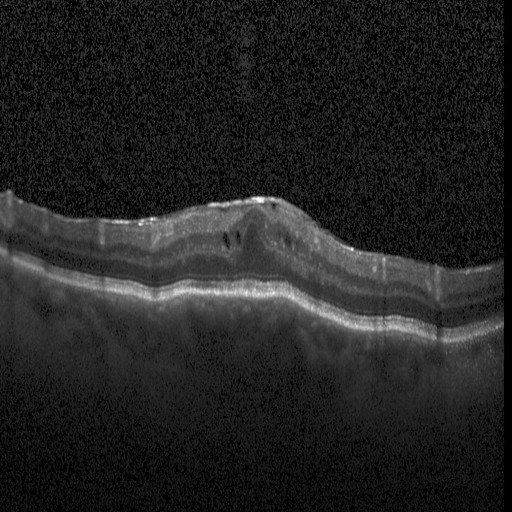

Optical coherence tomography B-scan
Impression: diabetic macular edema.